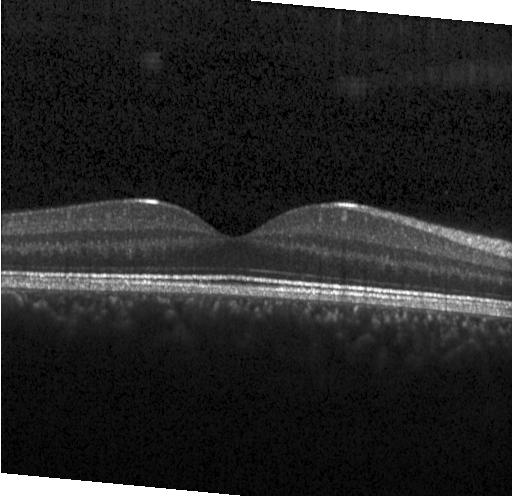 Optical coherence tomography scan, SD-OCT, through the macula.
Impression: no choroidal neovascularization, no diabetic macular edema, and no drusen.